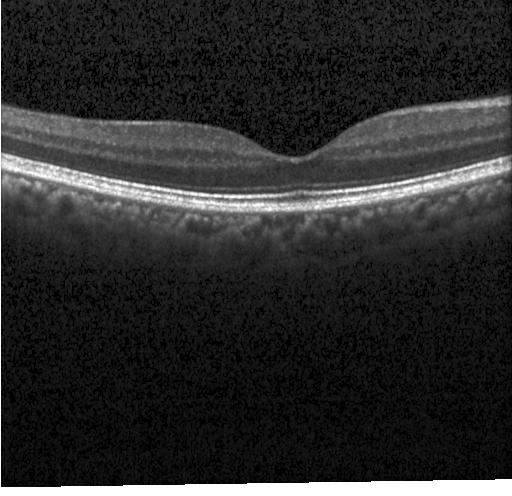 Spectral-domain optical coherence tomography. Retinal OCT B-scan. Macular scan. Instrument: Heidelberg Spectralis. Assessment: neither CNV, DME, nor drusen.